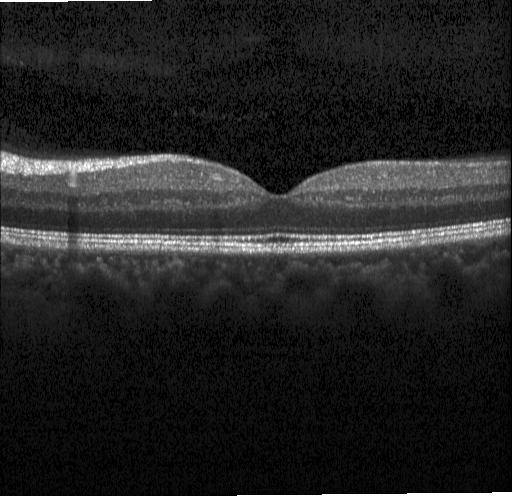
Spectral-domain optical coherence tomography. Acquired on a Heidelberg Spectralis. Through the macula. Optical coherence tomography B-scan
Macular OCT: no CNV, no DME, and no drusen.